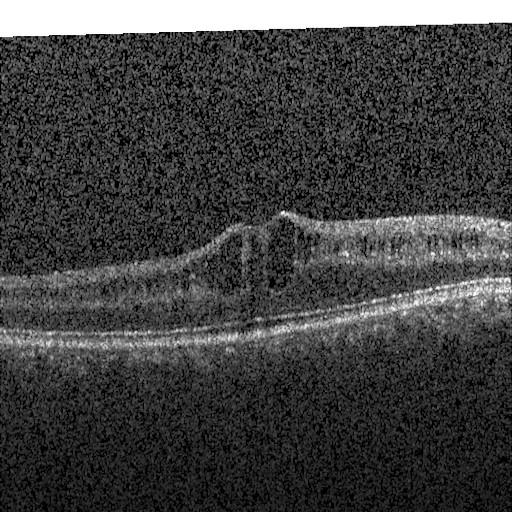 Impression: diabetic macular edema (DME).